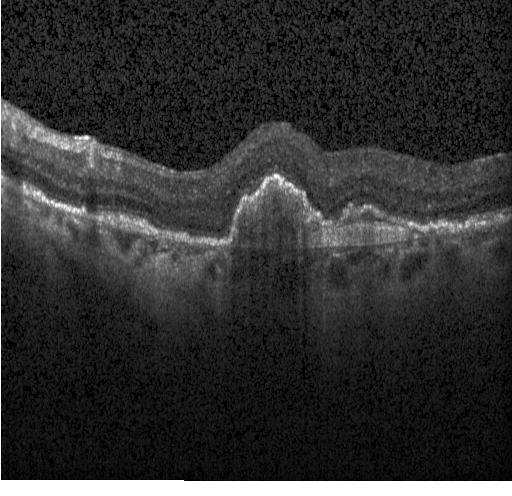
Assessment: a choroidal neovascular membrane.